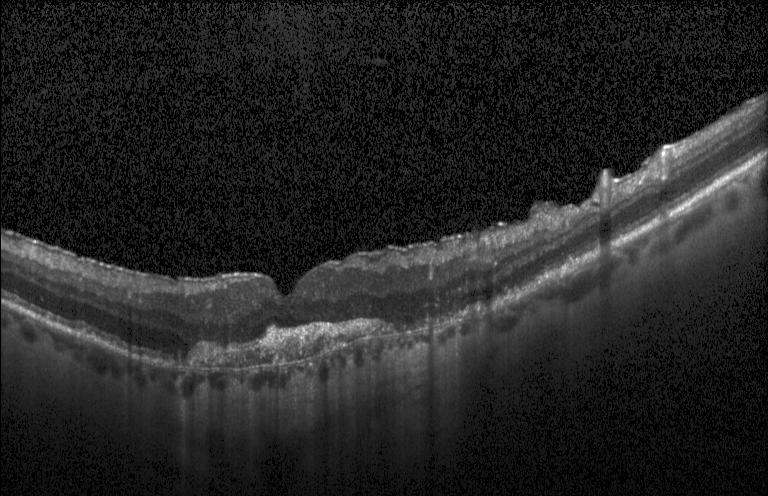 Optical coherence tomography B-scan — Diagnosis: CNV.